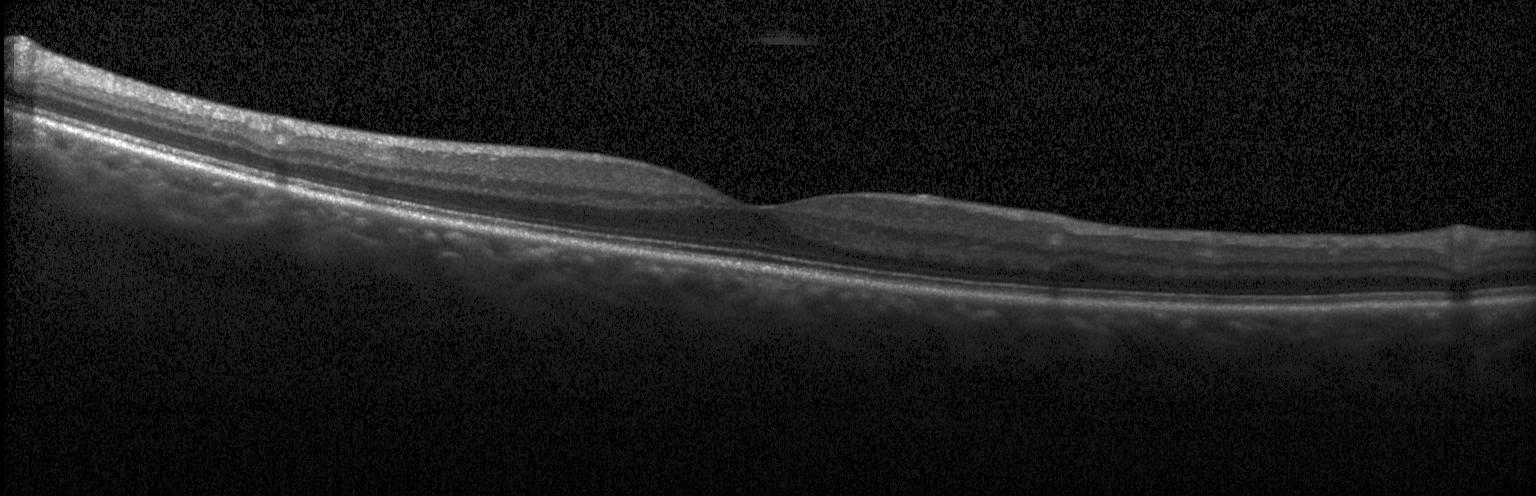
OCT B-scan showing no choroidal neovascularization, diabetic macular edema, or drusen.